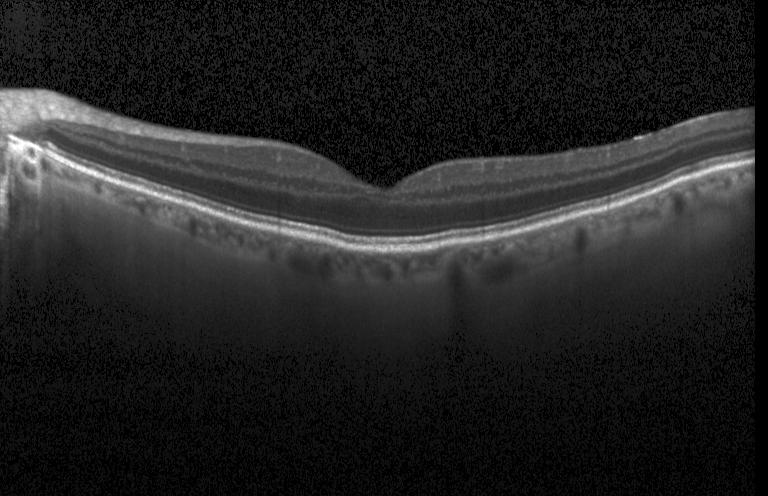
Spectral-domain OCT B-scan: no CNV, DME, or drusen.